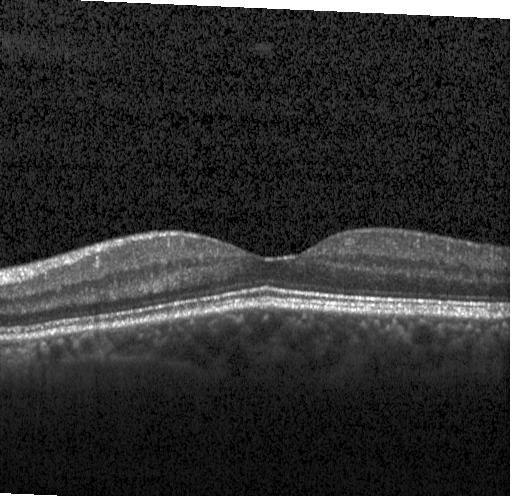 SD-OCT · Heidelberg Spectralis · horizontal scan through the fovea · optical coherence tomography B-scan. Diagnosis: no CNV, DME, or drusen.